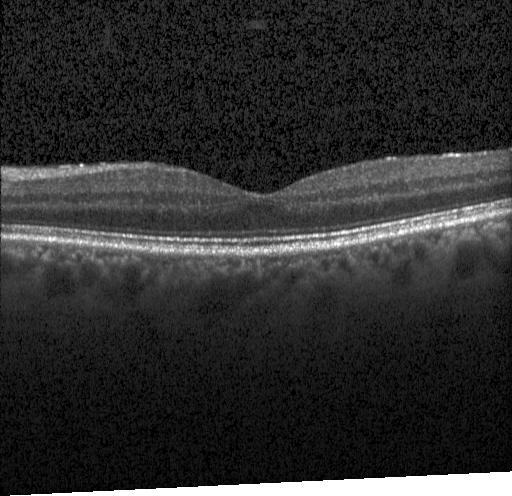 OCT line scan
OCT finding: no choroidal neovascularization, no diabetic macular edema, and no drusen.